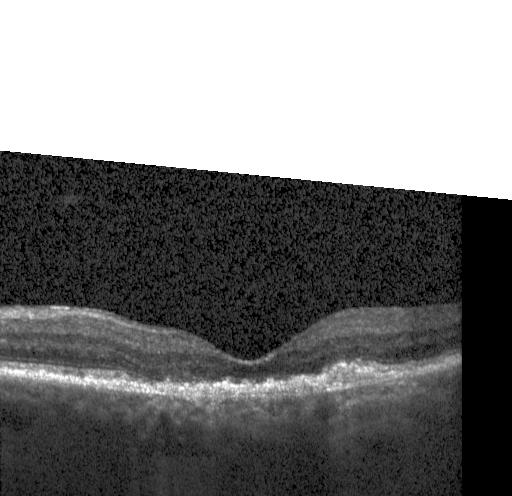 Heidelberg Spectralis OCT system, OCT B-scan. Finding: choroidal neovascularization.